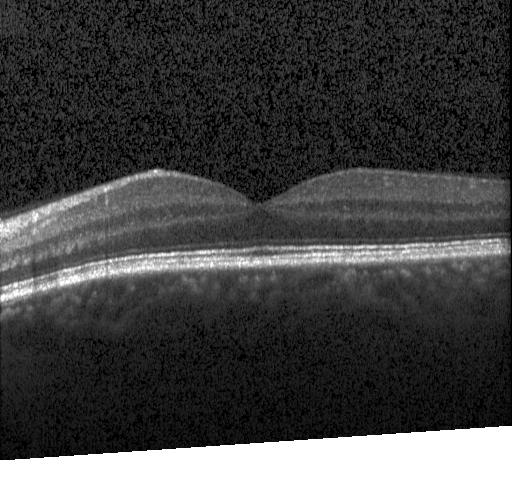 OCT B-scan · SD-OCT · acquired on a Heidelberg Spectralis — The scan shows no evidence of choroidal neovascularization, diabetic macular edema, or drusen.